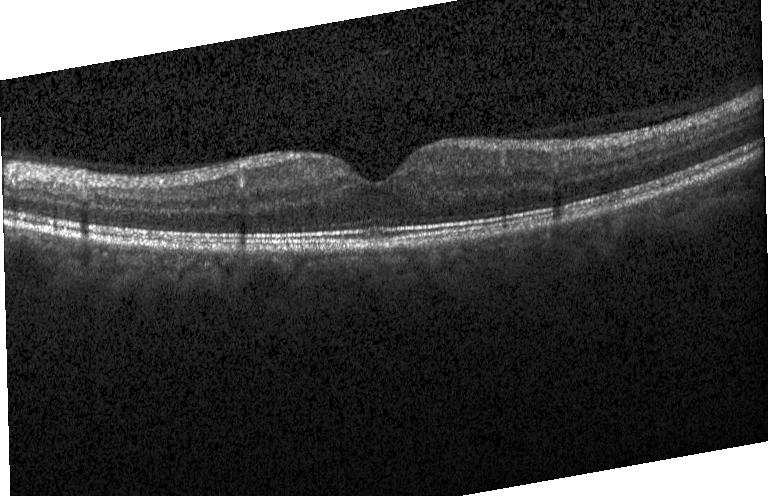
This B-scan demonstrates no choroidal neovascularization, no diabetic macular edema, and no drusen.